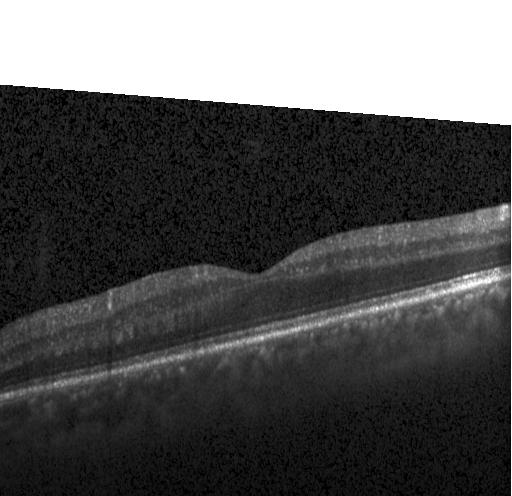 OCT B-scan.
Diagnosis: no evidence of CNV, DME, or drusen.